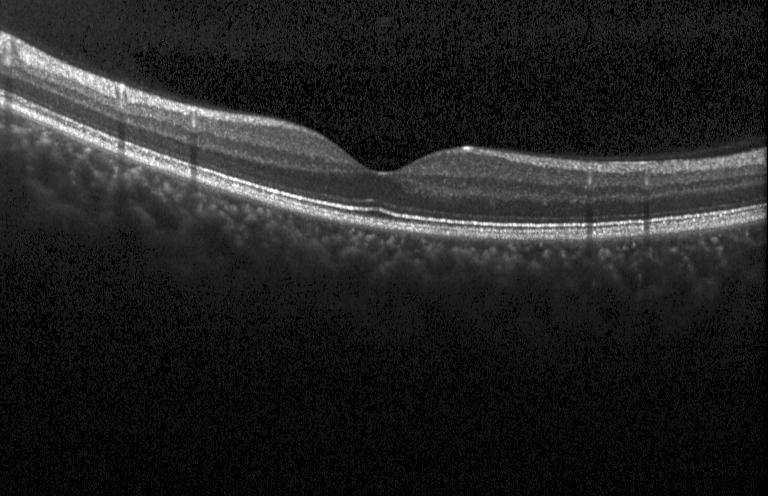 Retinal OCT B-scan, macular scan
Dx: no evidence of choroidal neovascularization, diabetic macular edema, or drusen.